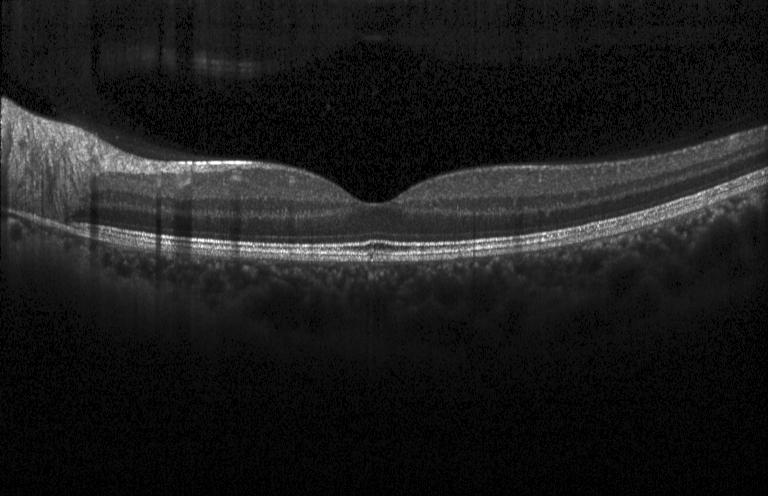

SD-OCT · retinal OCT B-scan. Impression: no evidence of choroidal neovascularization, diabetic macular edema, or drusen.